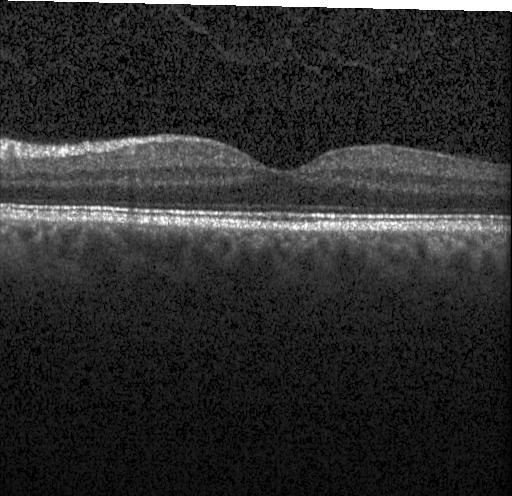 Horizontal scan through the fovea, Heidelberg Spectralis OCT system, OCT line scan, SD-OCT
Diagnosis: neither choroidal neovascularization, diabetic macular edema, nor drusen.